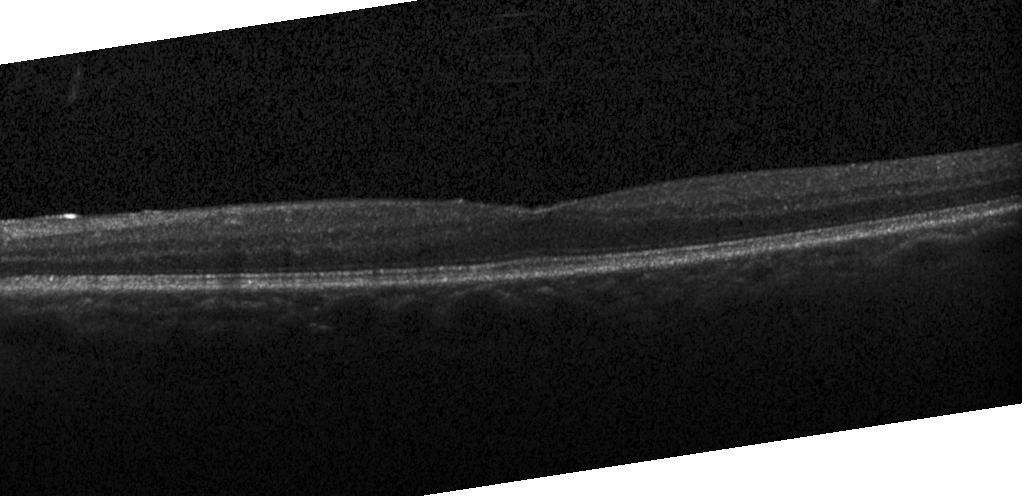 OCT B-scan, macular scan. The scan shows no evidence of choroidal neovascularization, diabetic macular edema, or drusen.